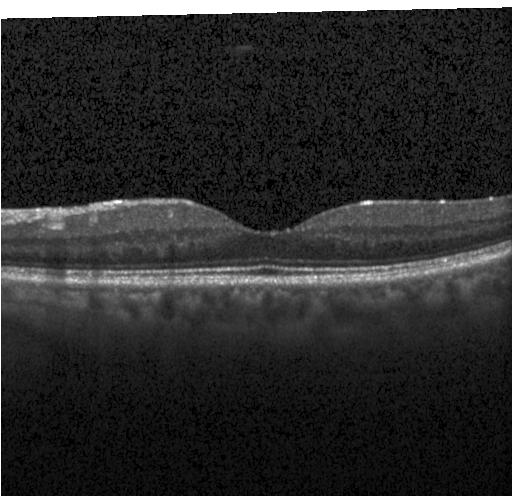
Optical coherence tomography B-scan.
Impression: no evidence of CNV, DME, or drusen.